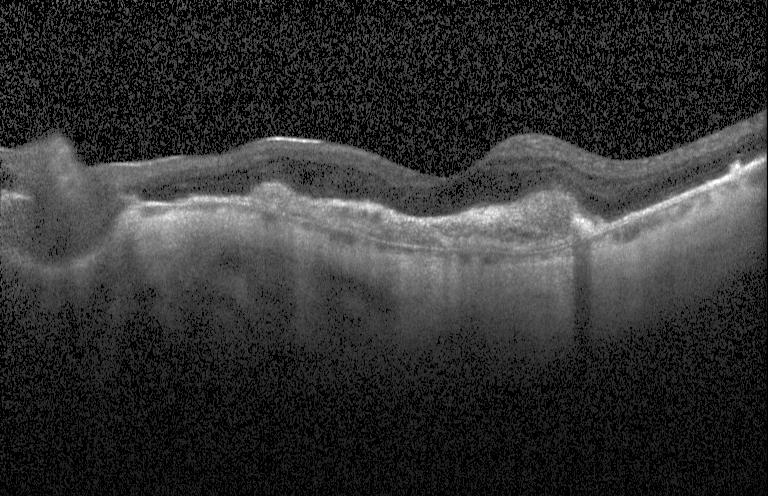

Horizontal scan through the fovea · spectral-domain OCT · optical coherence tomography B-scan — OCT finding: a choroidal neovascular membrane.